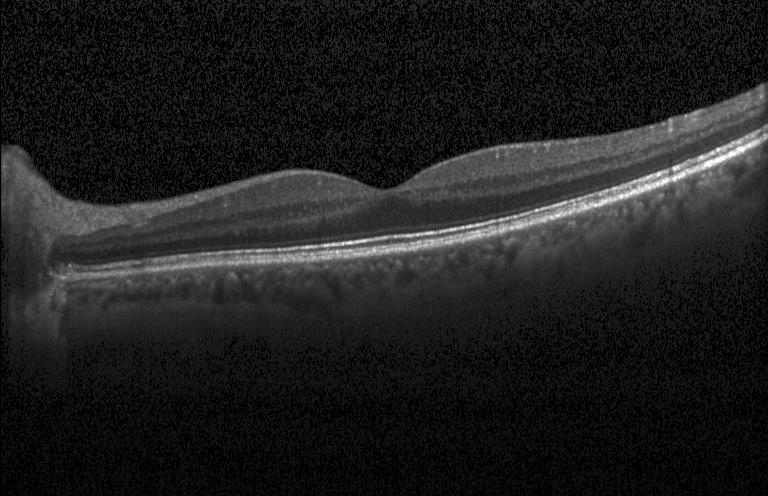 Acquired on a Heidelberg Spectralis, horizontal scan through the fovea, optical coherence tomography B-scan — Impression: no choroidal neovascularization, no diabetic macular edema, and no drusen.